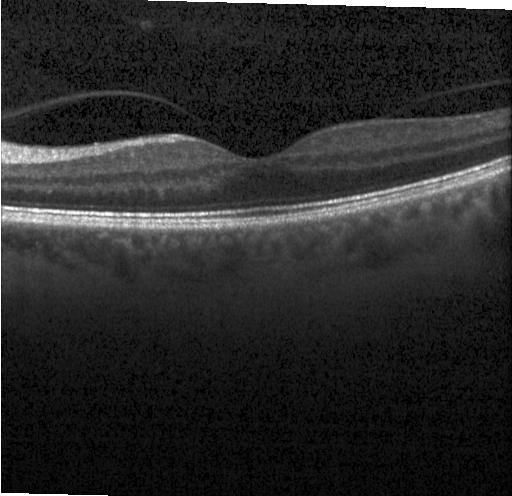

Retinal OCT cross-section. Acquired on a Heidelberg Spectralis. Spectral-domain OCT. Finding: no CNV, DME, or drusen.